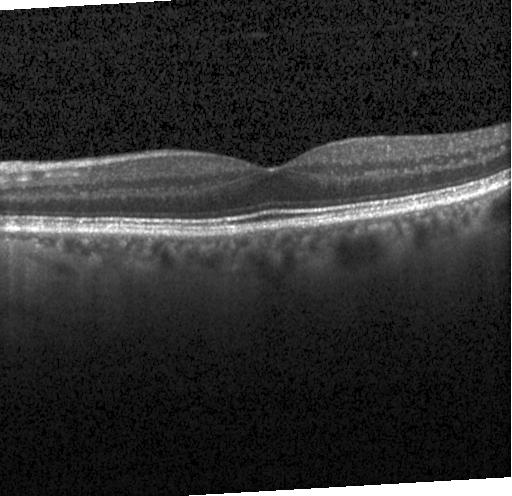 Optical coherence tomography B-scan
OCT finding: neither choroidal neovascularization, diabetic macular edema, nor drusen.